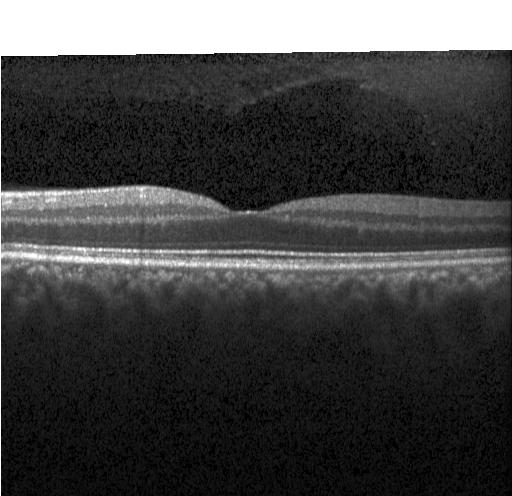 Optical coherence tomography scan.
OCT finding: neither choroidal neovascularization, diabetic macular edema, nor drusen.